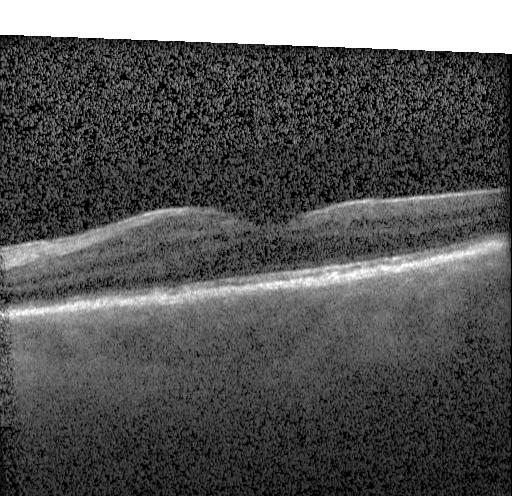
Macular OCT: neither choroidal neovascularization, diabetic macular edema, nor drusen.